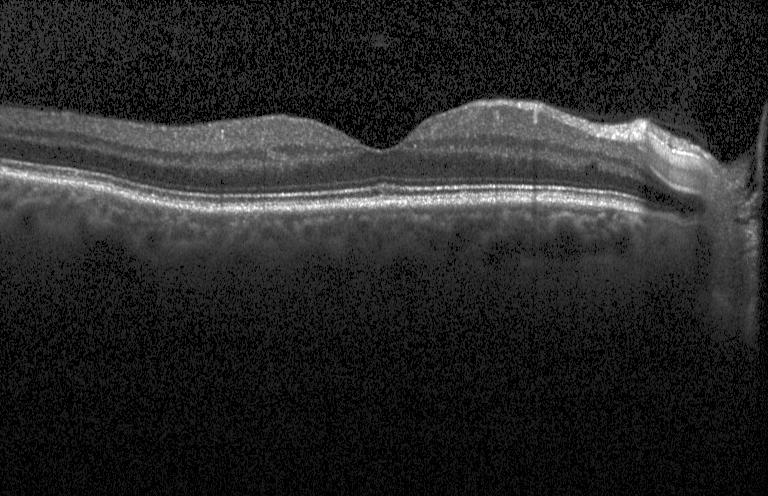 Dx: neither choroidal neovascularization, diabetic macular edema, nor drusen.